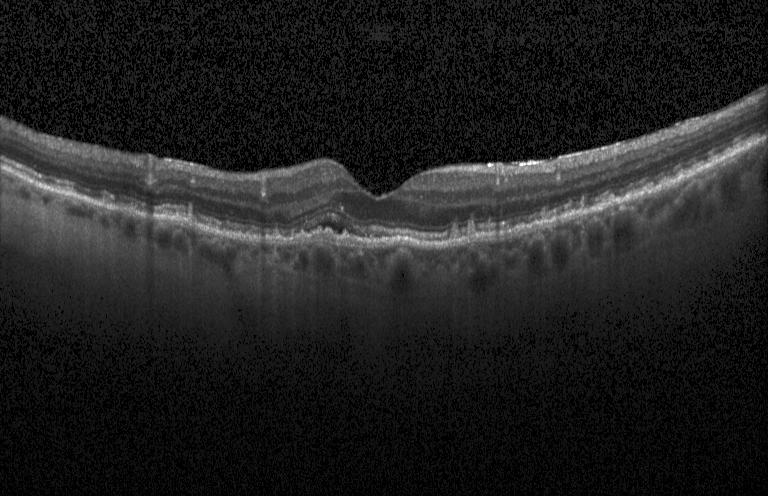 Impression: choroidal neovascularization.